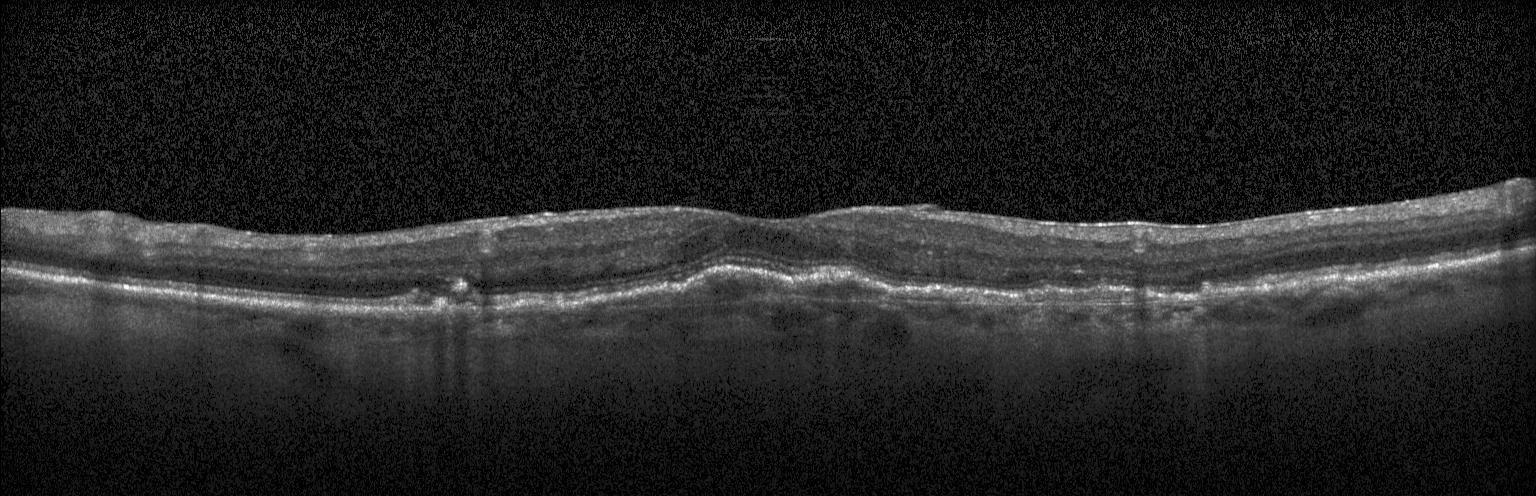
SD-OCT, acquired on a Heidelberg Spectralis, OCT line scan, centered on the fovea
Diagnosis: a choroidal neovascular membrane.